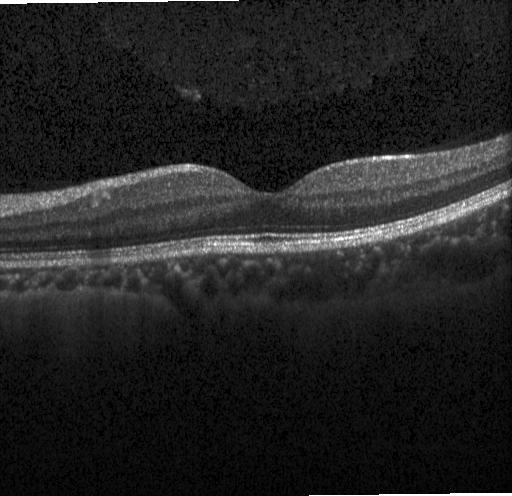 Spectral-domain optical coherence tomography · Heidelberg Spectralis · optical coherence tomography B-scan · centered on the fovea. The scan shows no CNV, no DME, and no drusen.